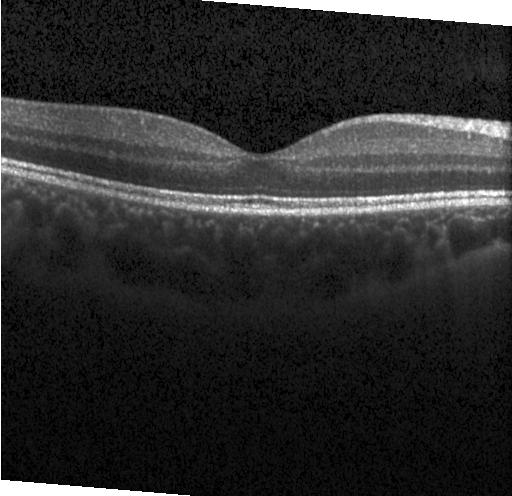

OCT scan showing no evidence of choroidal neovascularization, diabetic macular edema, or drusen.